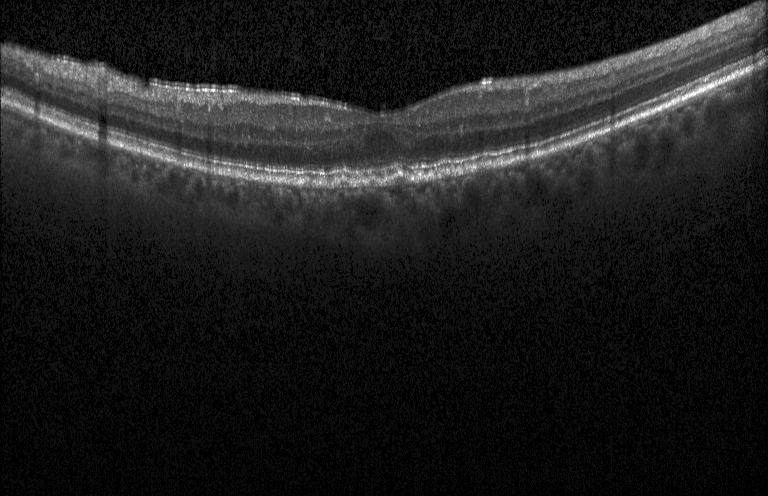 Spectral-domain OCT B-scan: sub-RPE drusenoid deposits.